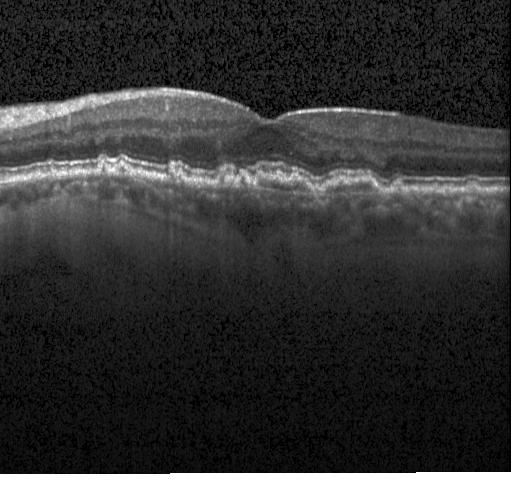

Heidelberg Spectralis OCT system. OCT line scan — This B-scan demonstrates multiple drusen.